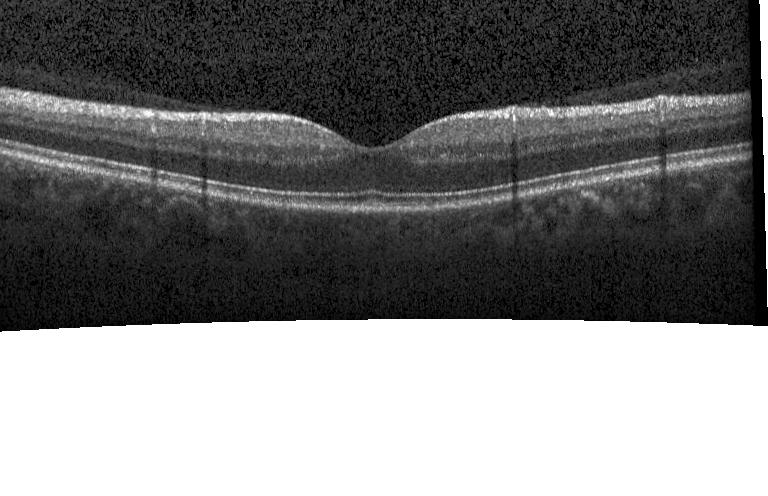

Assessment: no evidence of choroidal neovascularization, diabetic macular edema, or drusen.